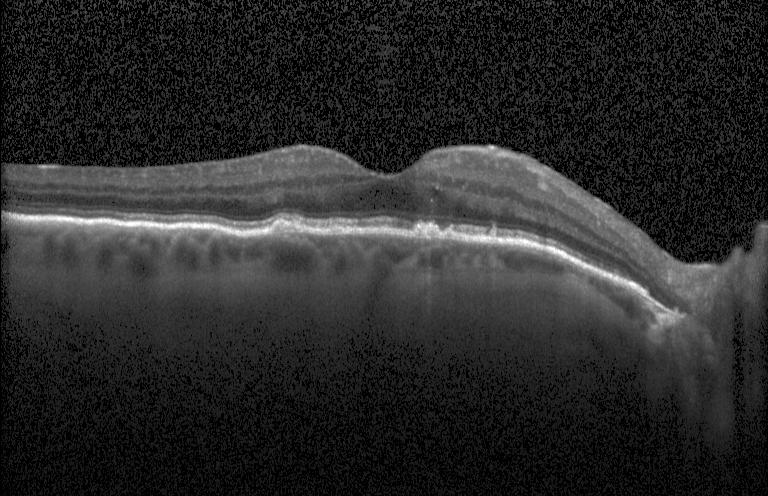
SD-OCT · optical coherence tomography scan · horizontal scan through the fovea. Drusen.